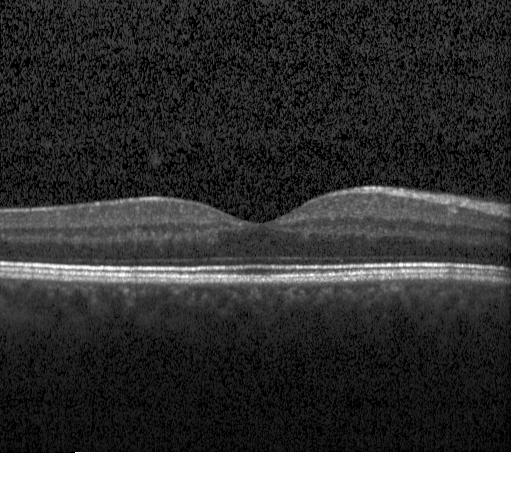
Impression: no choroidal neovascularization, no diabetic macular edema, and no drusen.